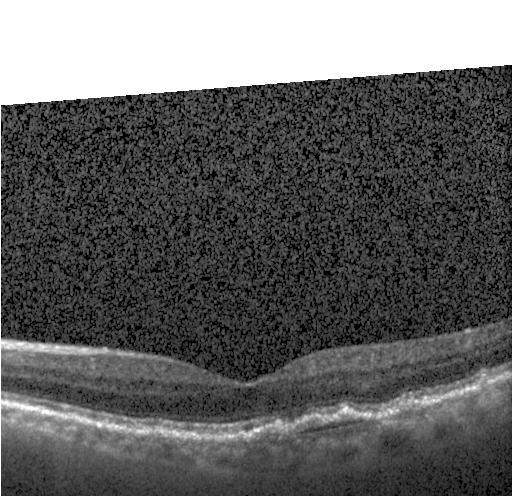 Spectral-domain OCT B-scan: choroidal neovascularization (CNV).